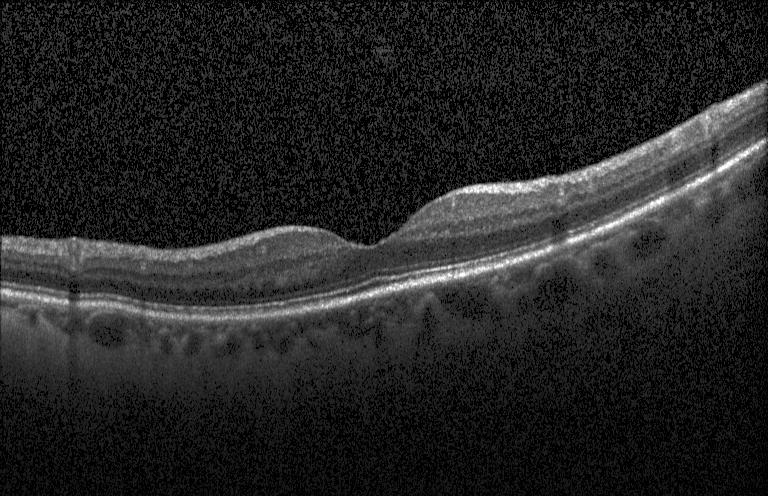 OCT finding: neither choroidal neovascularization, diabetic macular edema, nor drusen.